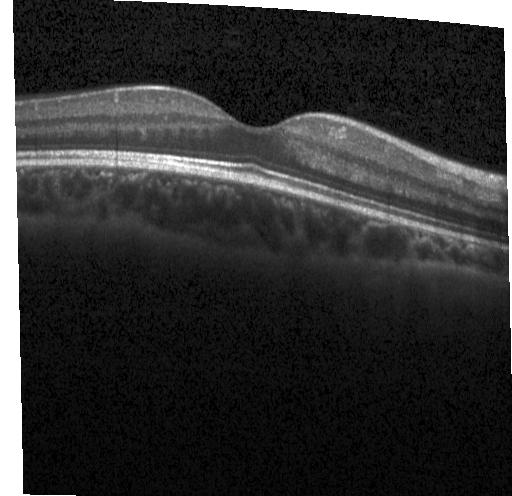
This B-scan demonstrates no choroidal neovascularization, diabetic macular edema, or drusen.